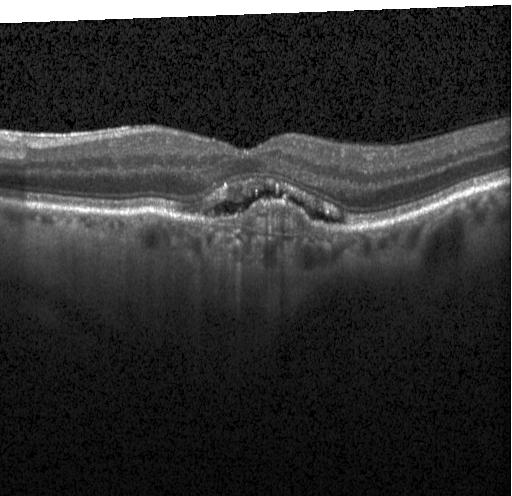

Acquired on a Heidelberg Spectralis, horizontal scan through the fovea, optical coherence tomography B-scan
Choroidal neovascularization.